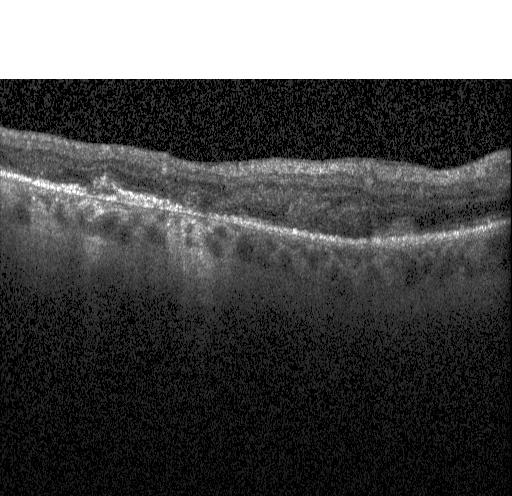
Horizontal scan through the fovea. Retinal OCT B-scan. SD-OCT. Heidelberg Spectralis.
Macular OCT: choroidal neovascularization.